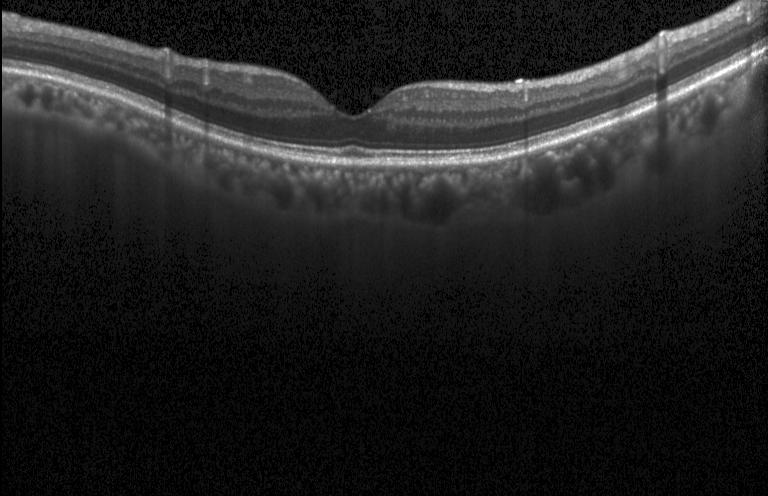
Retinal OCT B-scan
Neither choroidal neovascularization, diabetic macular edema, nor drusen.